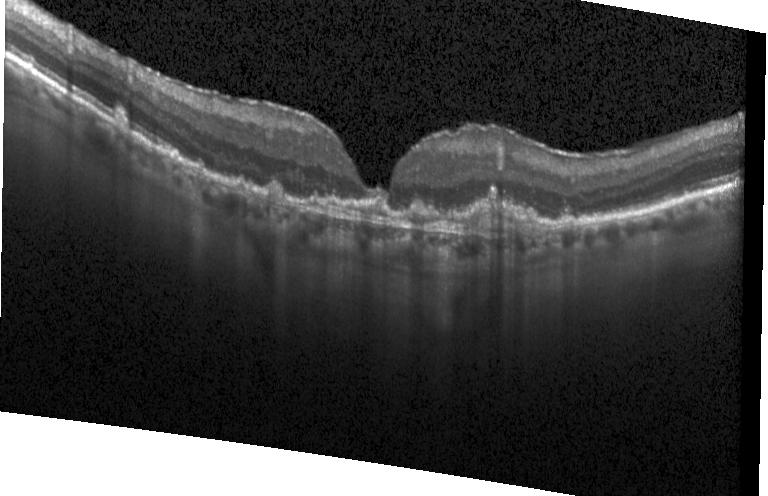

Spectral-domain OCT B-scan: choroidal neovascularization.